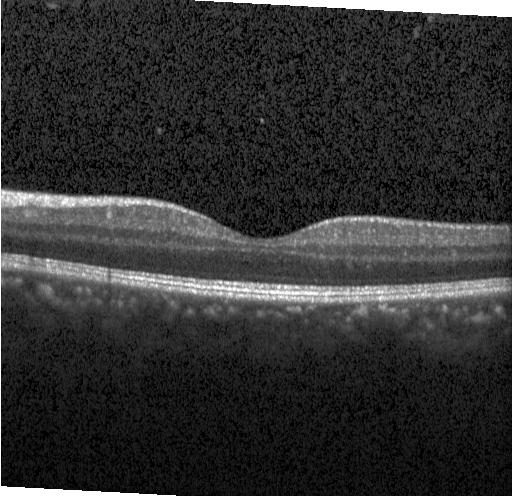

Through the macula. Optical coherence tomography B-scan. SD-OCT.
Finding: no choroidal neovascularization, no diabetic macular edema, and no drusen.